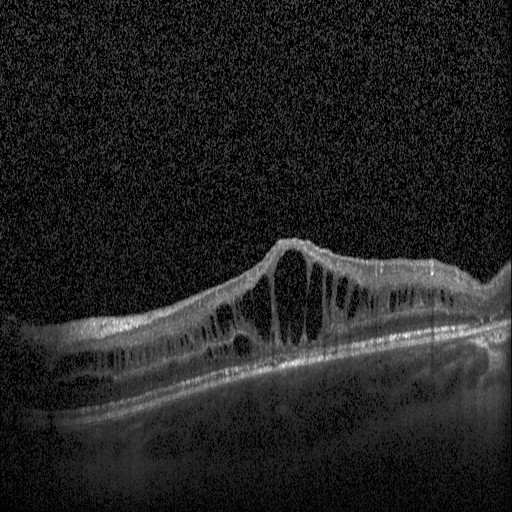

Instrument: Heidelberg Spectralis; retinal OCT B-scan; fovea-centered; spectral-domain optical coherence tomography — Macular OCT: diabetic macular edema.